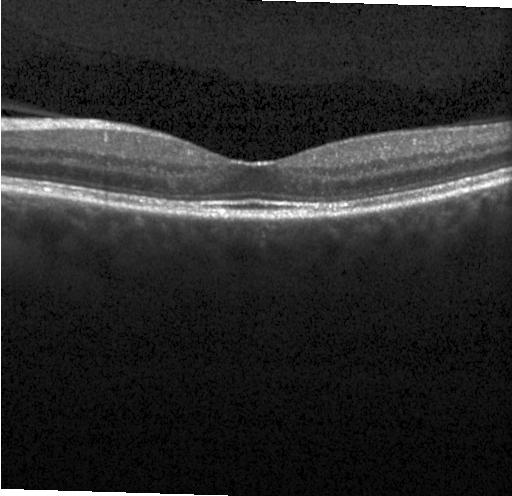
Optical coherence tomography scan
The scan shows no choroidal neovascularization, diabetic macular edema, or drusen.